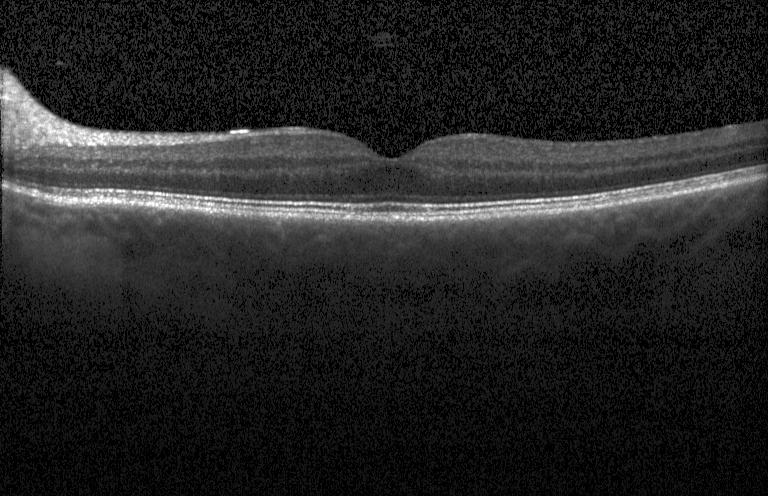
No evidence of choroidal neovascularization, diabetic macular edema, or drusen.